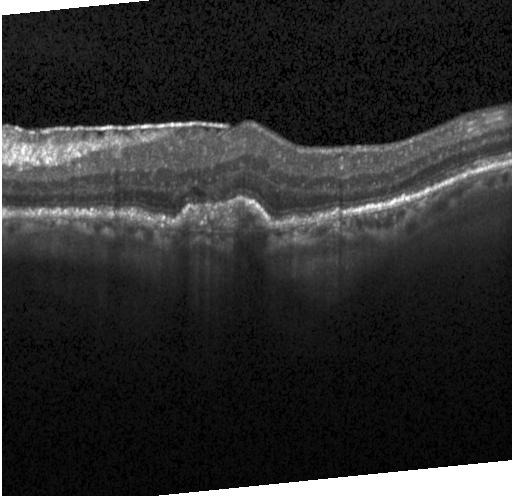
OCT B-scan; through the macula; SD-OCT. Diagnosis: choroidal neovascularization (CNV).